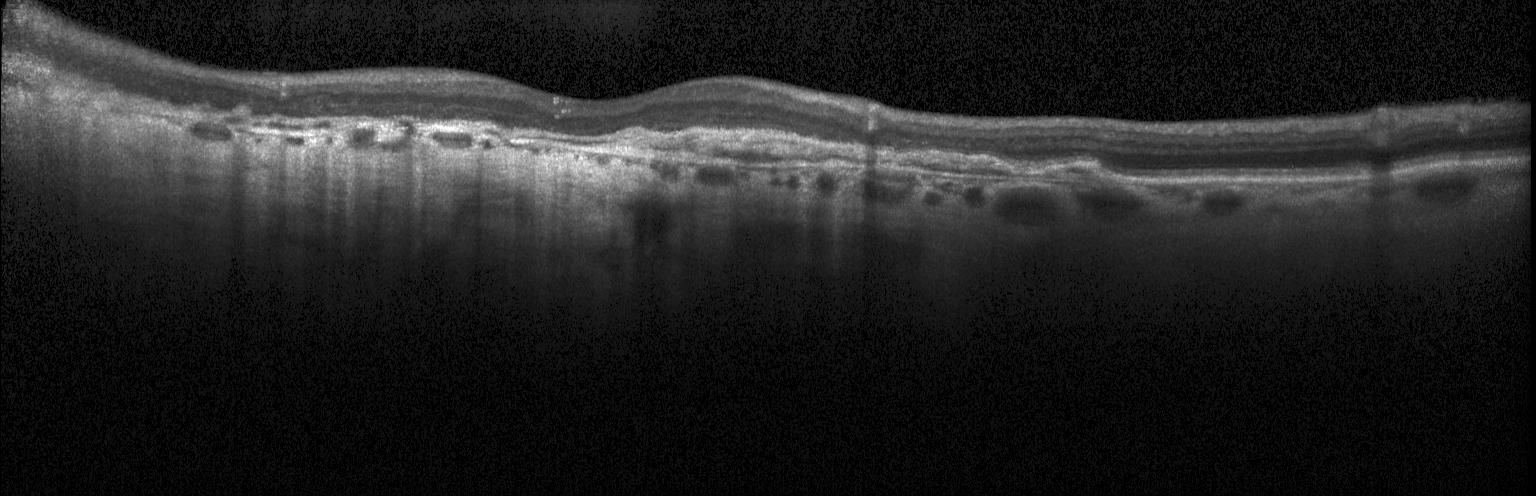 This B-scan demonstrates choroidal neovascularization.